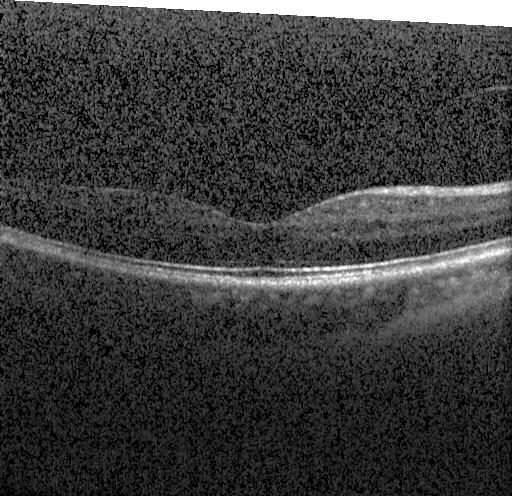

Optical coherence tomography B-scan
The scan shows no CNV, no DME, and no drusen.